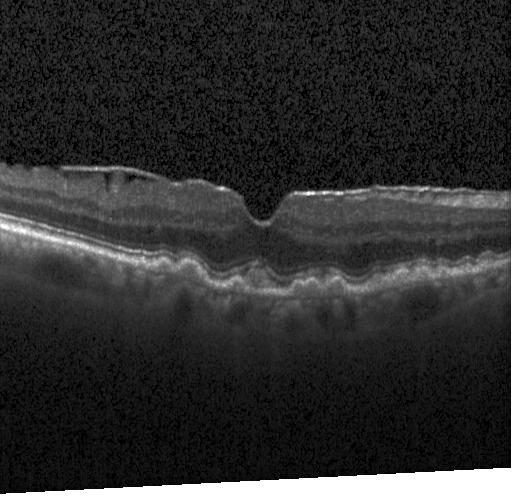

Heidelberg Spectralis; through the macula; OCT B-scan
Assessment: sub-RPE drusenoid deposits.